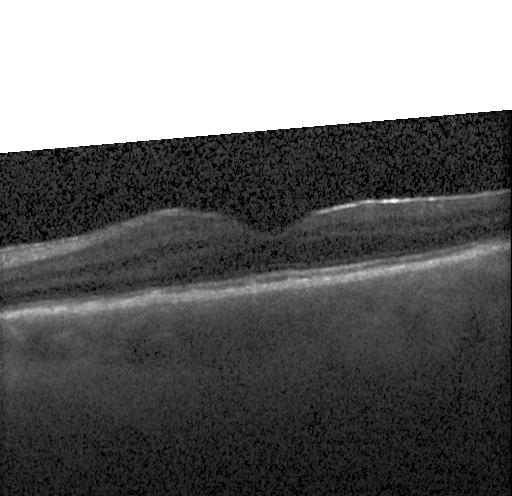
Spectral-domain OCT B-scan: no evidence of CNV, DME, or drusen.